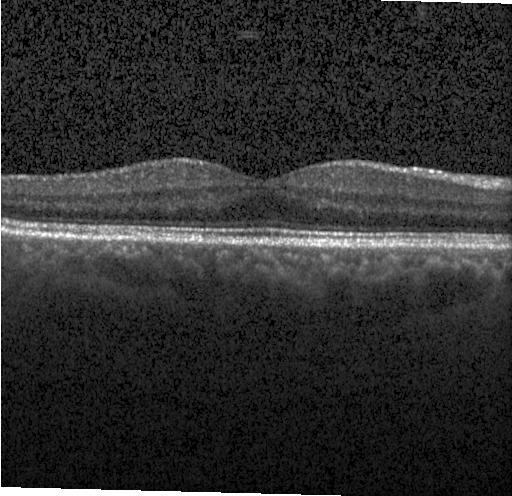
Macular scan. Heidelberg Spectralis OCT system. Spectral-domain OCT. Retinal OCT cross-section
Assessment: no CNV, DME, or drusen.